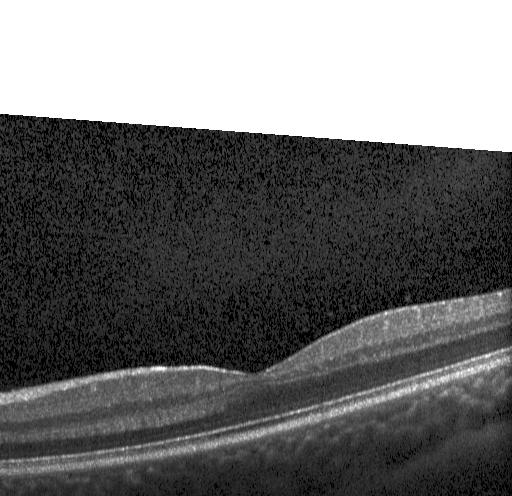
OCT finding: no CNV, no DME, and no drusen.